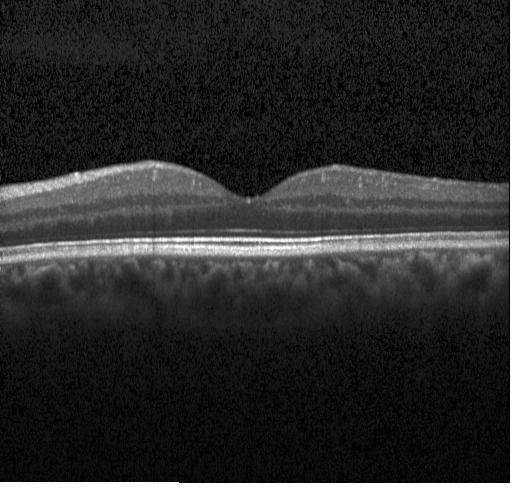 Optical coherence tomography B-scan, Heidelberg Spectralis OCT system, spectral-domain optical coherence tomography — Macular OCT: no choroidal neovascularization, diabetic macular edema, or drusen.